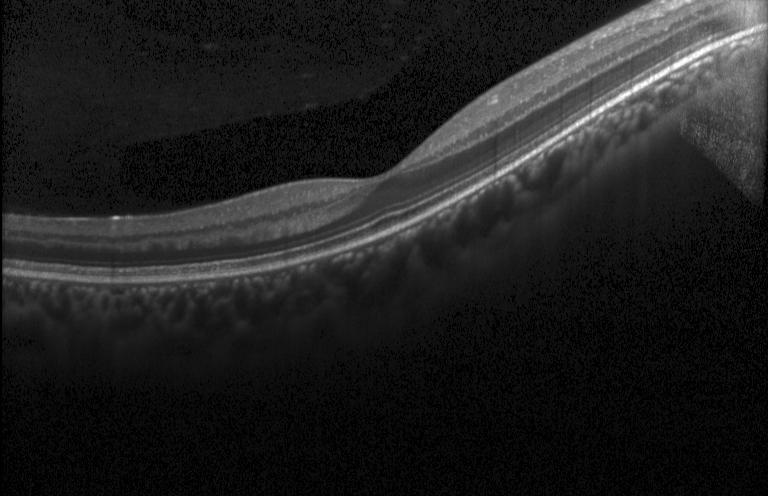 OCT line scan.
Dx: no choroidal neovascularization, diabetic macular edema, or drusen.